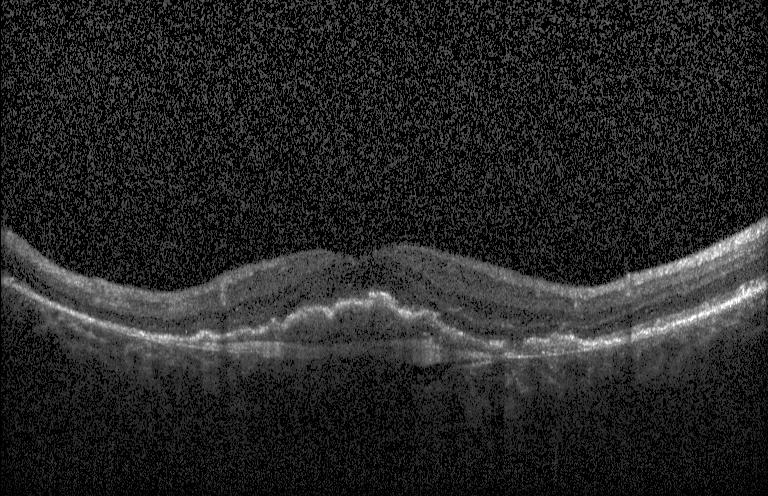 Fovea-centered. OCT B-scan — Impression: a choroidal neovascular membrane.